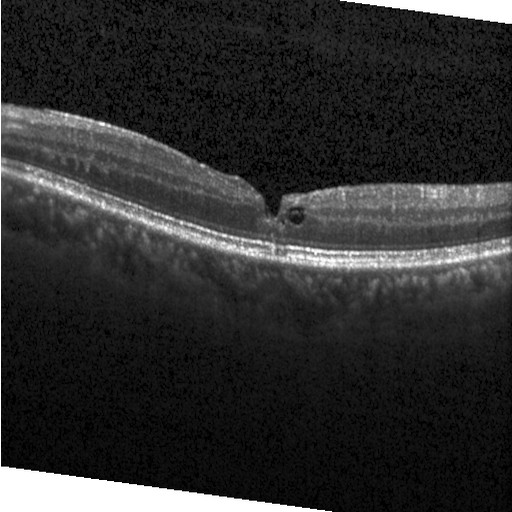 SD-OCT, acquired on a Heidelberg Spectralis, OCT B-scan, macular scan.
Macular OCT: diabetic macular edema.